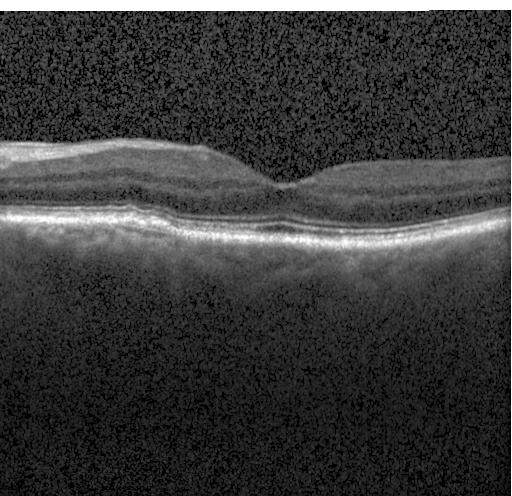
Retinal OCT cross-section showing sub-RPE drusenoid deposits.